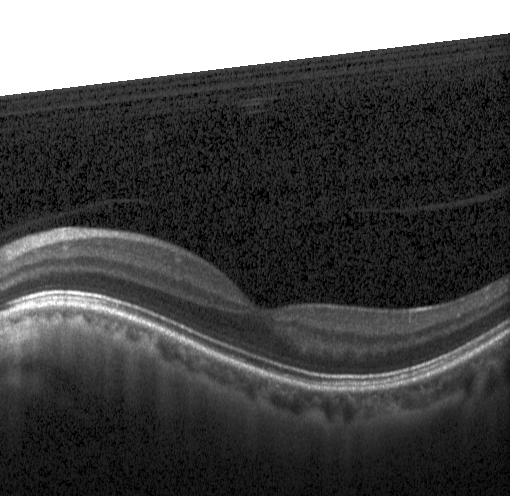

OCT scan showing no CNV, no DME, and no drusen.